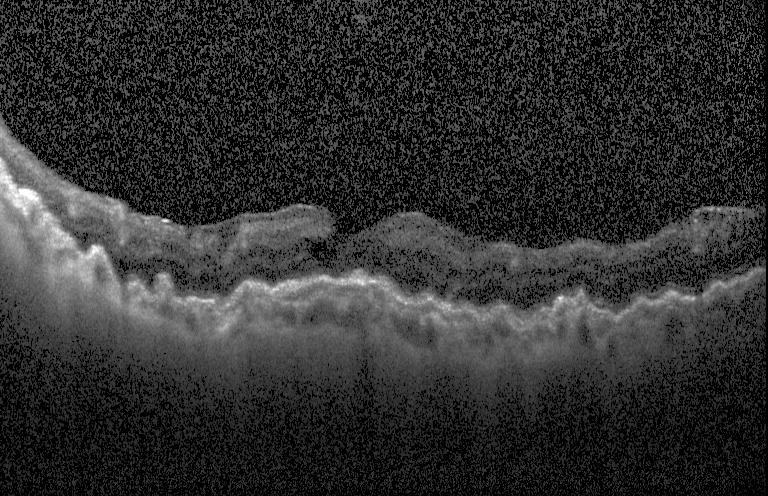
OCT B-scan, macular scan, spectral-domain optical coherence tomography. This B-scan demonstrates CNV.